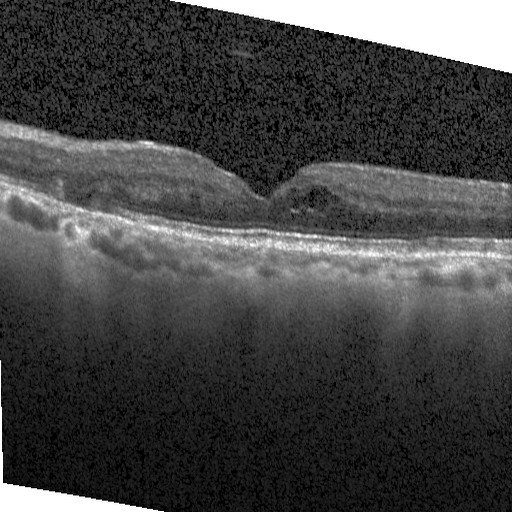

Retinal OCT cross-section; macular scan; Heidelberg Spectralis OCT system; SD-OCT
Diagnosis: diabetic macular edema.